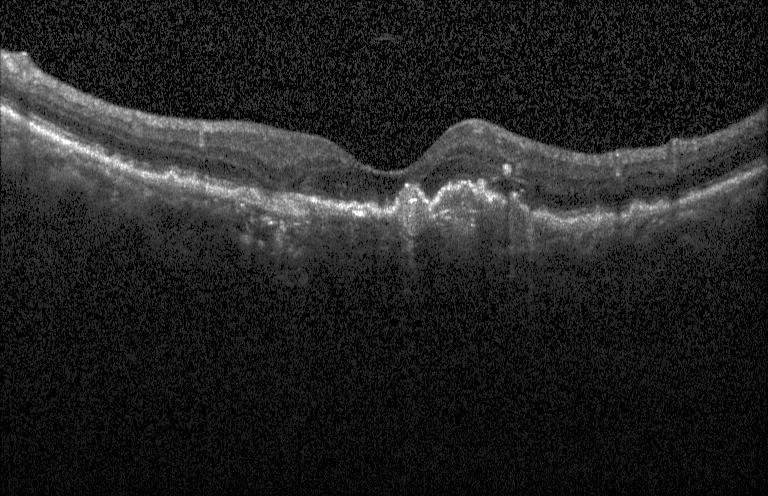
Optical coherence tomography B-scan. Spectral-domain OCT. Horizontal scan through the fovea — The scan shows choroidal neovascularization.